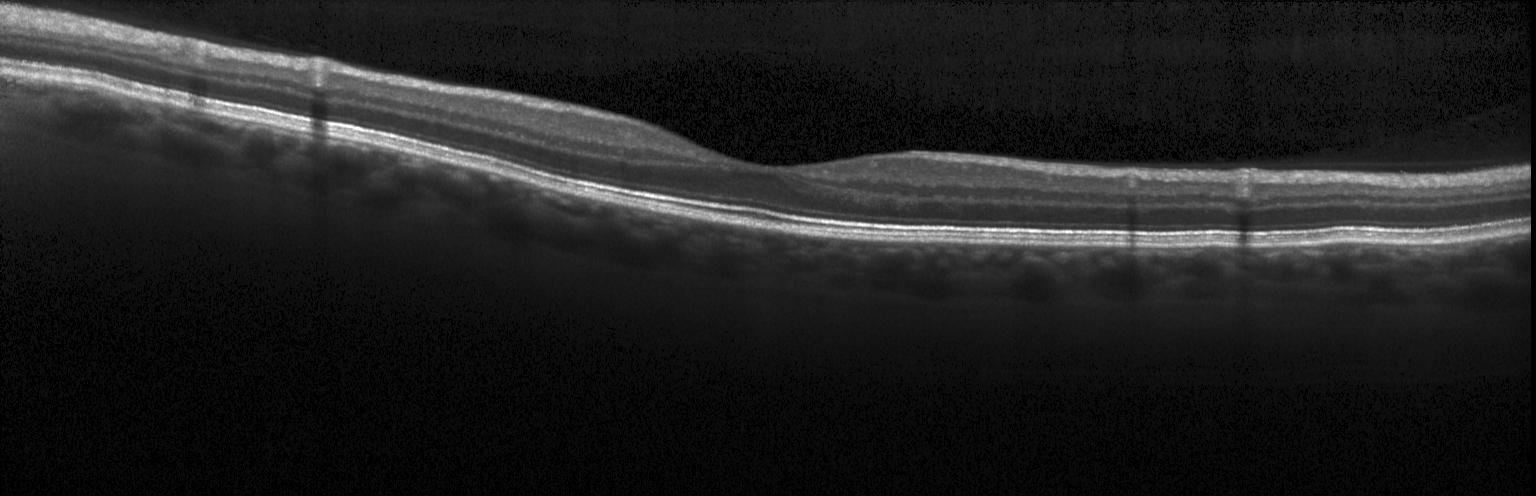
OCT B-scan; Heidelberg Spectralis; spectral-domain OCT; centered on the fovea. Finding: no choroidal neovascularization, no diabetic macular edema, and no drusen.